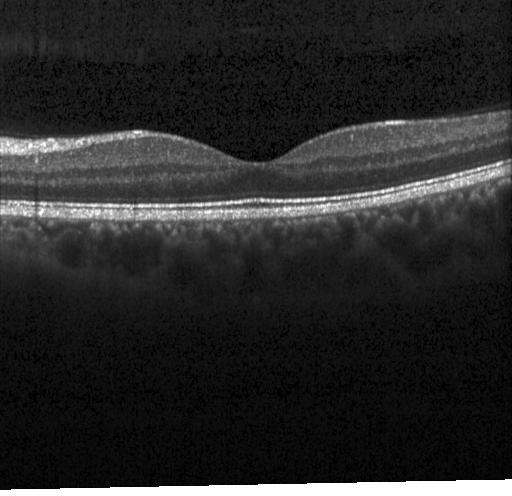
Retinal OCT B-scan. Spectral-domain OCT. Macular scan. Macular OCT: no evidence of CNV, DME, or drusen.